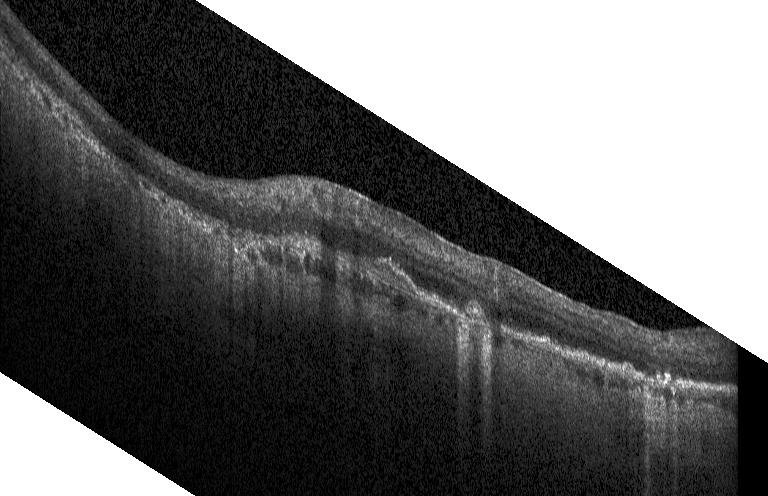 Horizontal scan through the fovea. Spectral-domain optical coherence tomography. Heidelberg Spectralis. Optical coherence tomography scan.
Choroidal neovascularization (CNV).